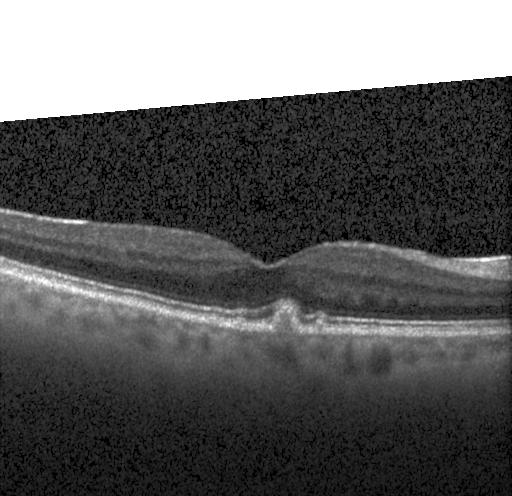
Through the macula. Heidelberg Spectralis. Optical coherence tomography B-scan. Spectral-domain optical coherence tomography
Macular OCT: drusen.